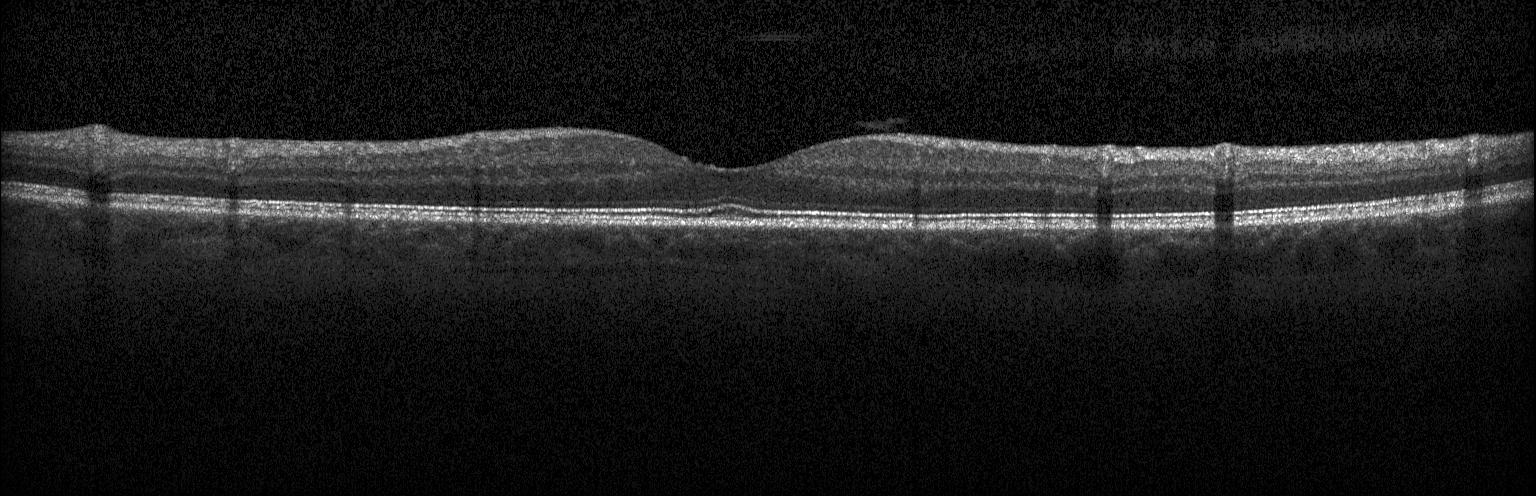 Impression: no CNV, DME, or drusen.